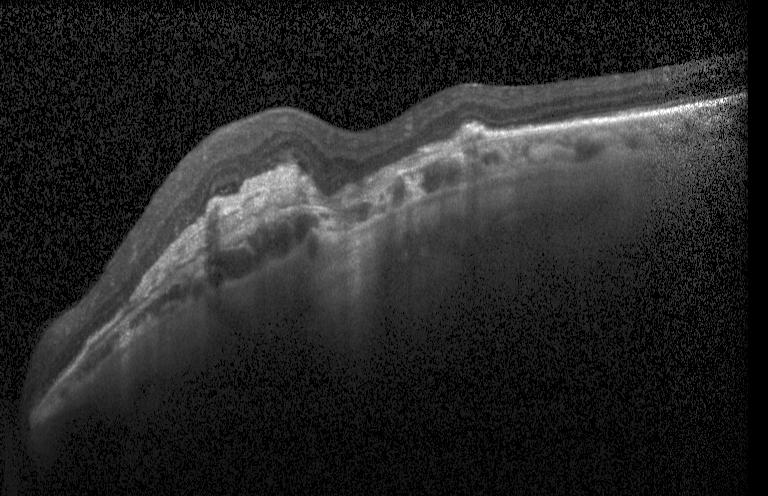

Acquired on a Heidelberg Spectralis. Retinal OCT cross-section — Macular OCT: choroidal neovascularization (CNV).